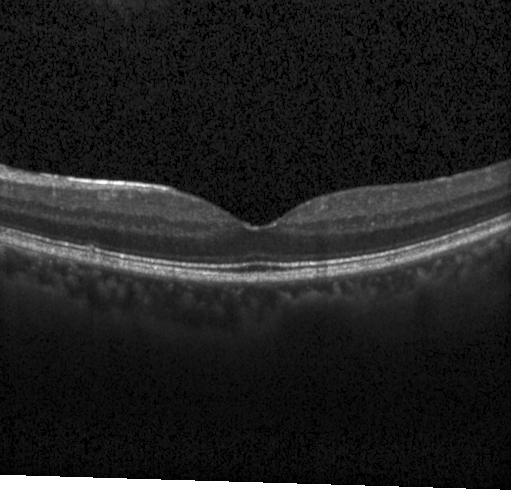
SD-OCT. Optical coherence tomography scan. OCT finding: no choroidal neovascularization, no diabetic macular edema, and no drusen.